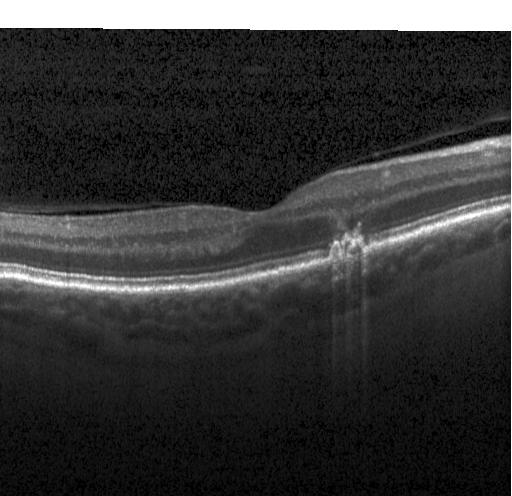

Spectral-domain OCT B-scan: sub-RPE drusenoid deposits.